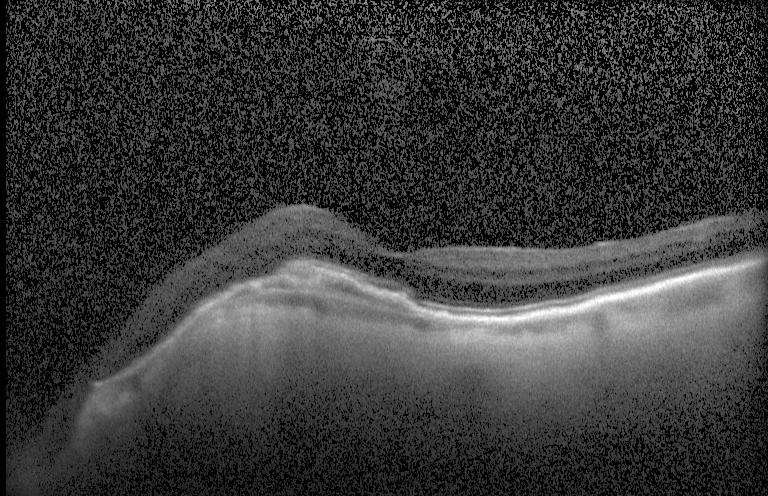
Retinal OCT cross-section showing a choroidal neovascular membrane.